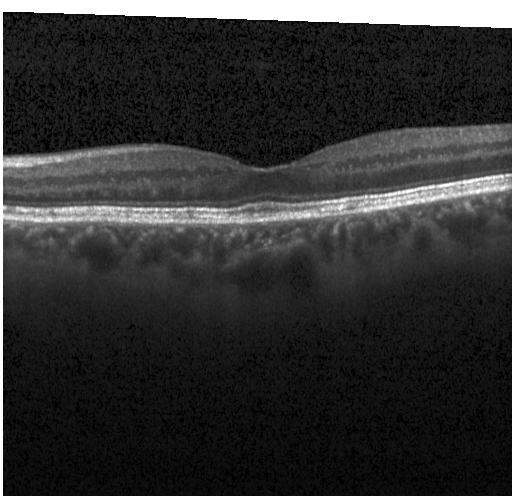 Optical coherence tomography scan, SD-OCT, instrument: Heidelberg Spectralis
This B-scan demonstrates no evidence of choroidal neovascularization, diabetic macular edema, or drusen.